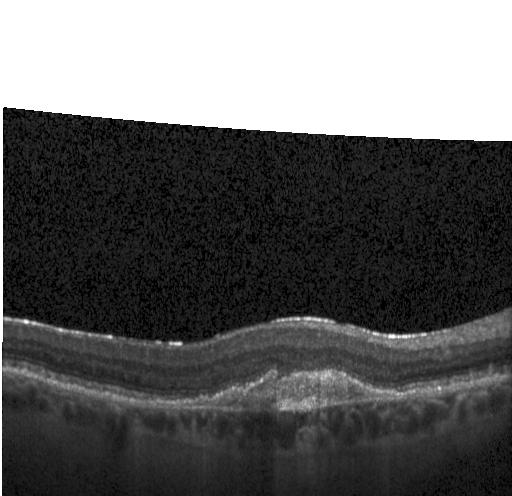

Spectral-domain OCT · optical coherence tomography B-scan · Heidelberg Spectralis OCT system · centered on the fovea — Macular OCT: CNV.